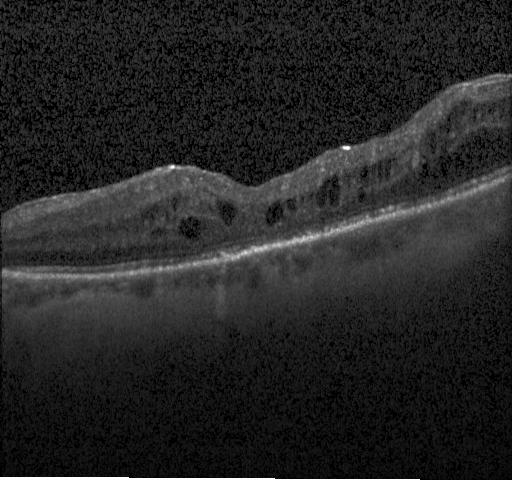 SD-OCT · horizontal scan through the fovea · retinal OCT cross-section. Diagnosis: diabetic macular edema.